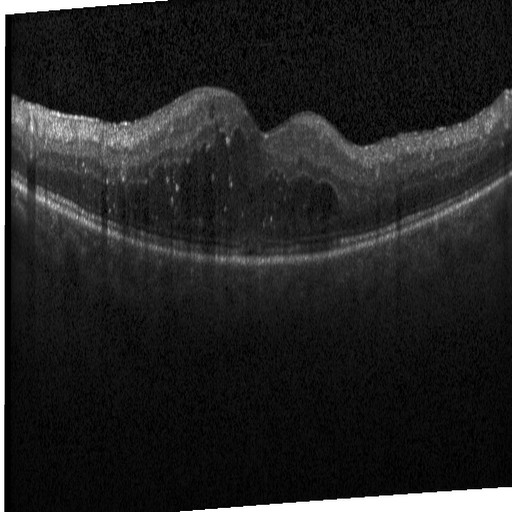

Diagnosis: diabetic macular edema.